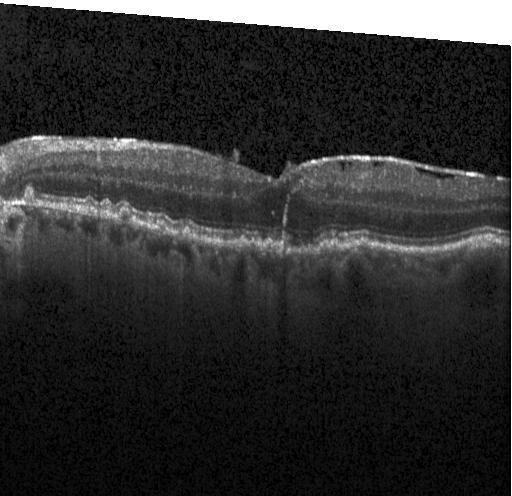
Macular OCT: sub-RPE drusenoid deposits.